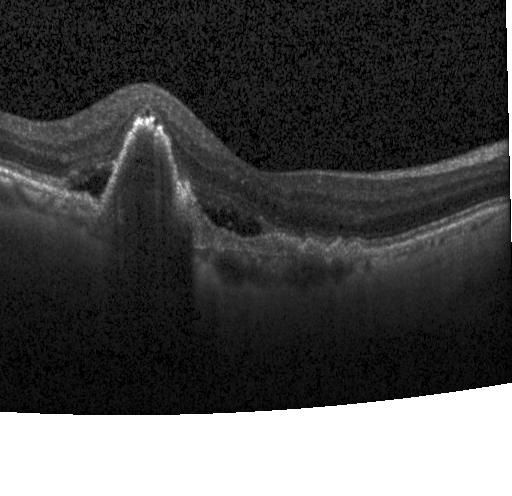 OCT line scan; through the macula; spectral-domain OCT. Diagnosis: CNV.